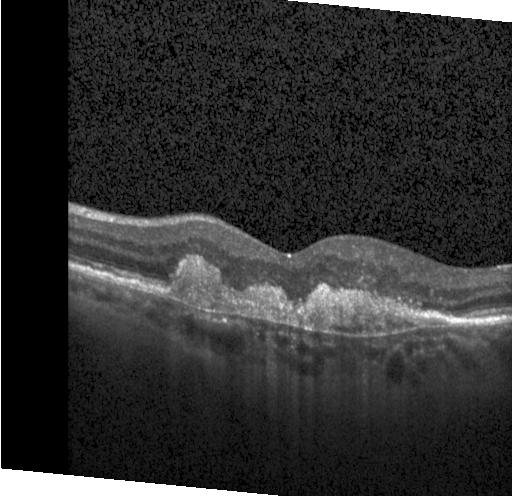
Macular scan. Retinal OCT cross-section. Spectral-domain optical coherence tomography. Heidelberg Spectralis OCT system. Impression: CNV.